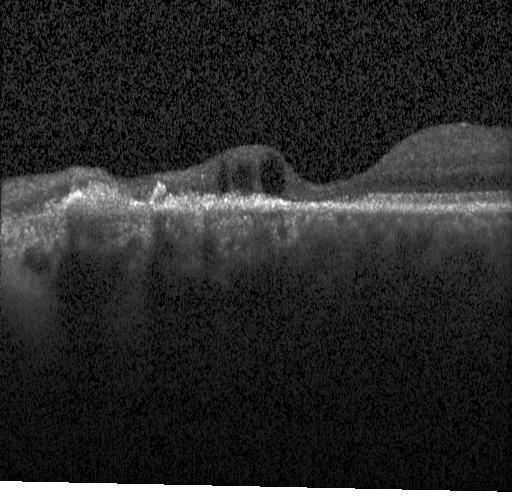 Spectral-domain OCT; OCT B-scan; instrument: Heidelberg Spectralis; fovea-centered — OCT finding: CNV.